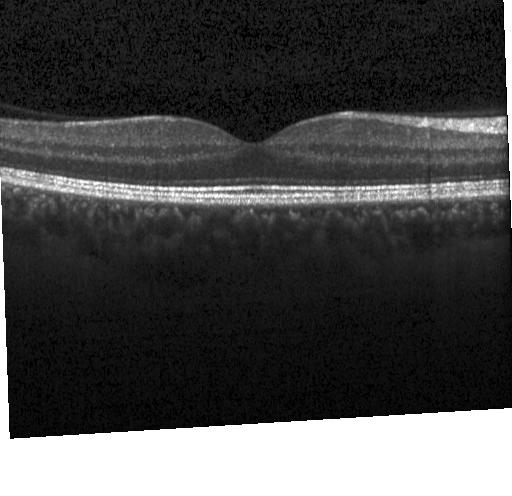
OCT line scan. Finding: no evidence of CNV, DME, or drusen.